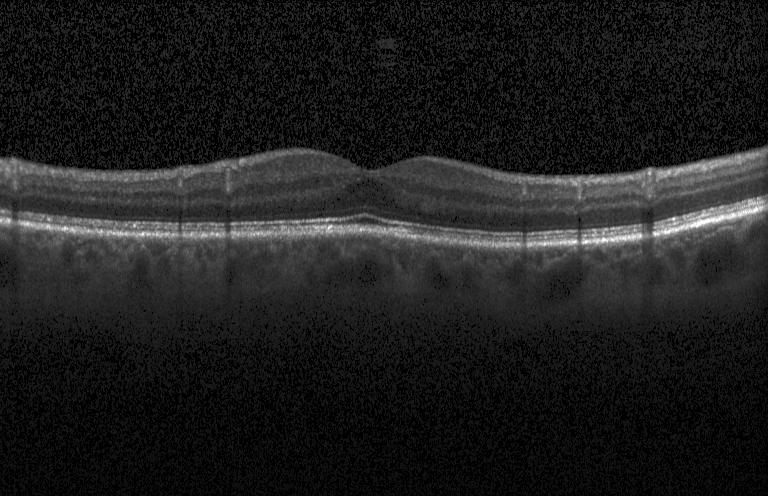
Instrument: Heidelberg Spectralis; optical coherence tomography scan; macular scan — Neither choroidal neovascularization, diabetic macular edema, nor drusen.